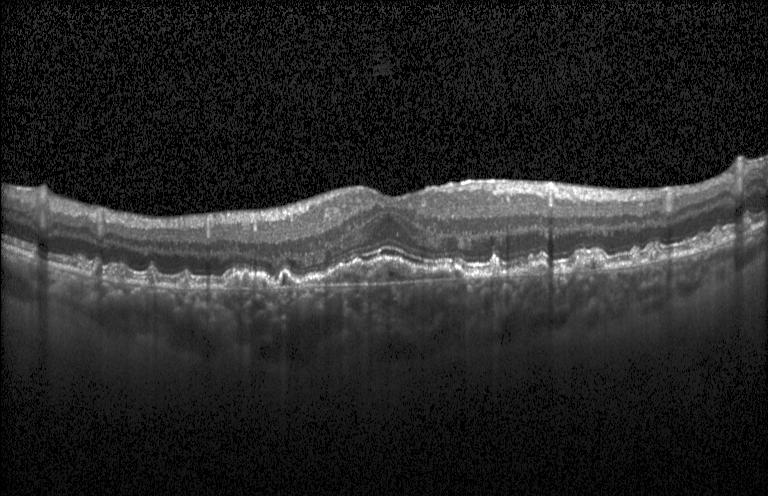 SD-OCT; centered on the fovea; OCT B-scan; Heidelberg Spectralis OCT system.
Dx: a choroidal neovascular membrane.